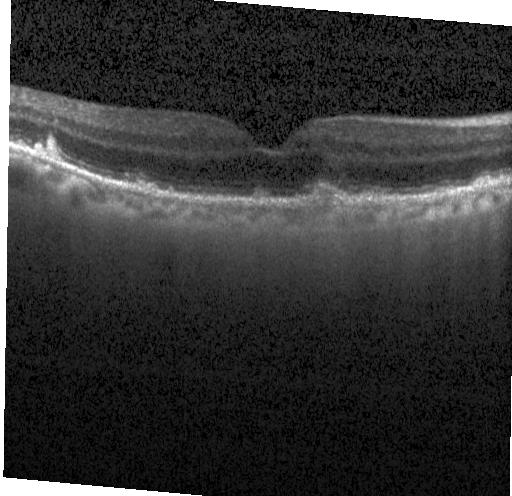

Sub-RPE drusenoid deposits.